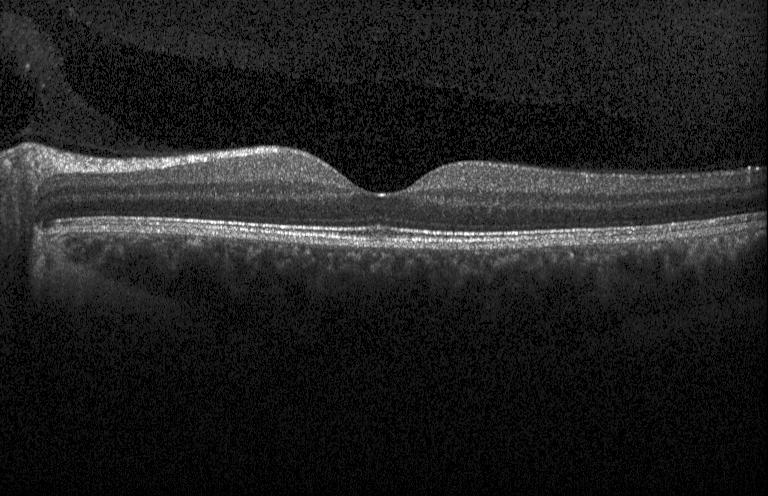 This B-scan demonstrates neither choroidal neovascularization, diabetic macular edema, nor drusen.